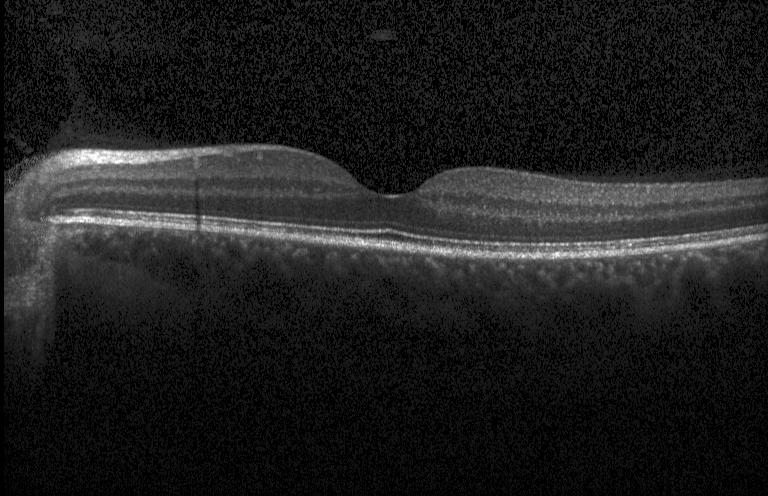 Spectral-domain optical coherence tomography. OCT B-scan. Through the macula. Acquired on a Heidelberg Spectralis
Dx: no evidence of CNV, DME, or drusen.